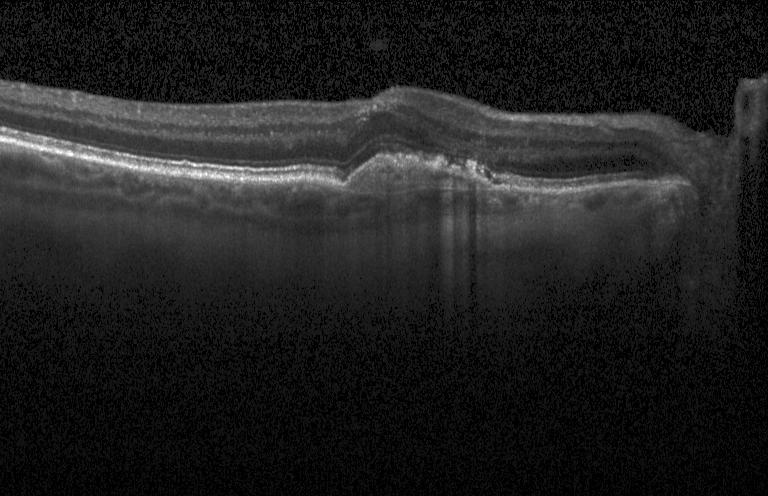
OCT line scan · SD-OCT — Dx: a choroidal neovascular membrane.